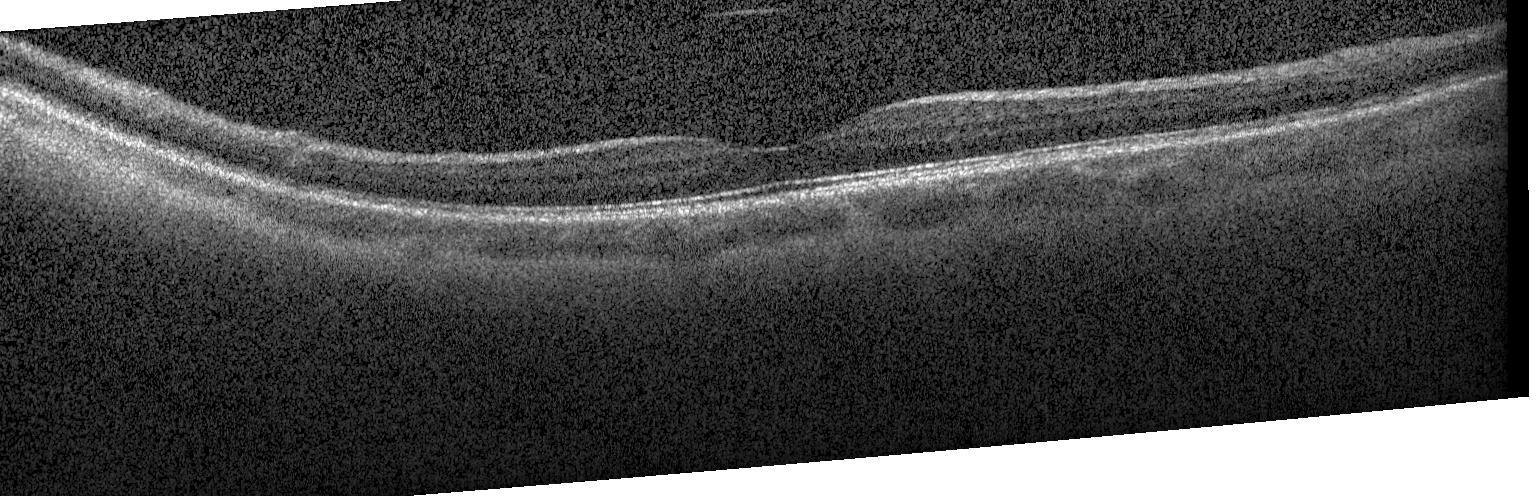
Macular OCT: neither choroidal neovascularization, diabetic macular edema, nor drusen.